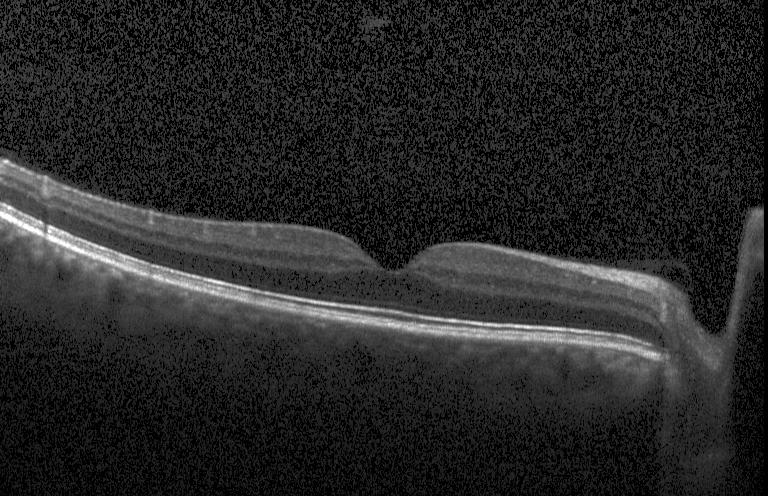
OCT B-scan. Macular scan. Spectral-domain OCT
Finding: no choroidal neovascularization, diabetic macular edema, or drusen.